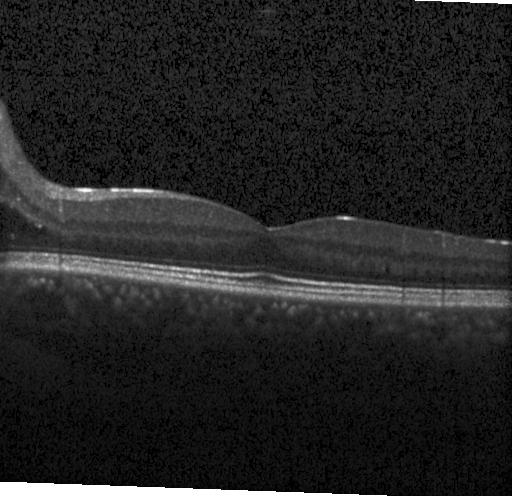

OCT finding: no choroidal neovascularization, diabetic macular edema, or drusen.